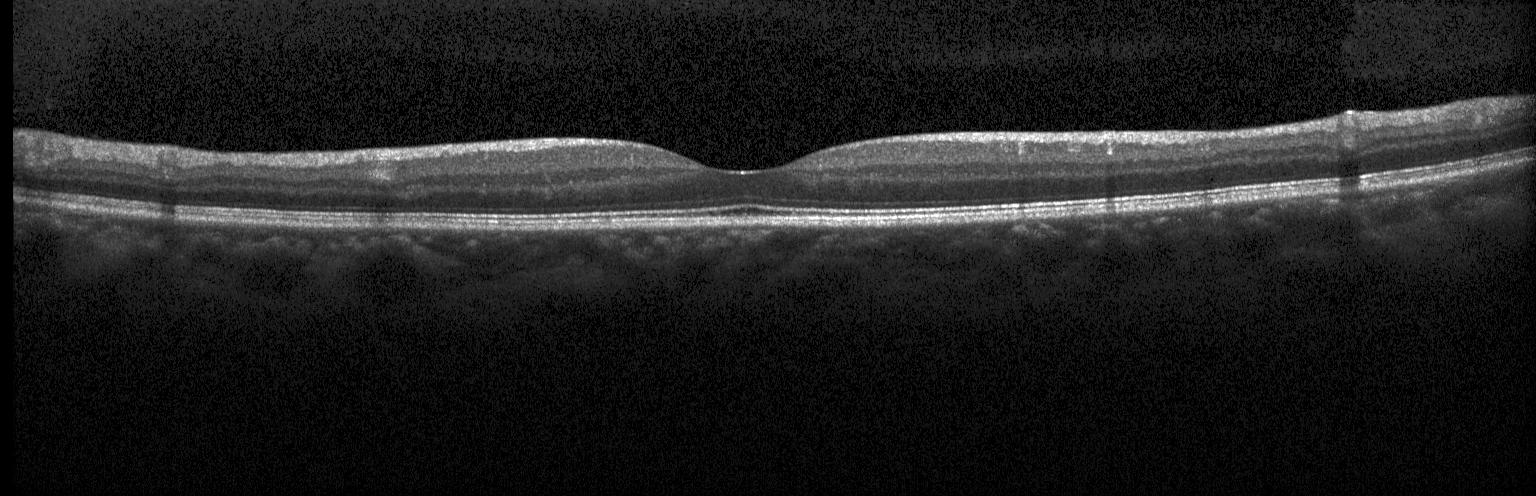 Optical coherence tomography B-scan — Dx: neither choroidal neovascularization, diabetic macular edema, nor drusen.